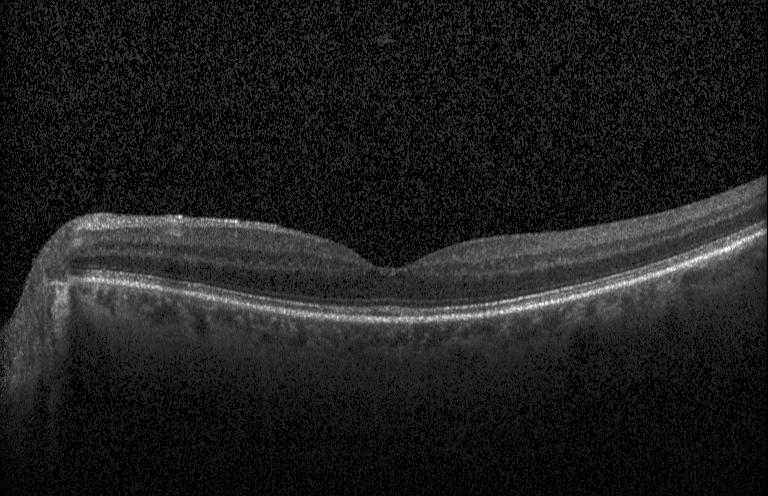
OCT B-scan — Diagnosis: neither CNV, DME, nor drusen.